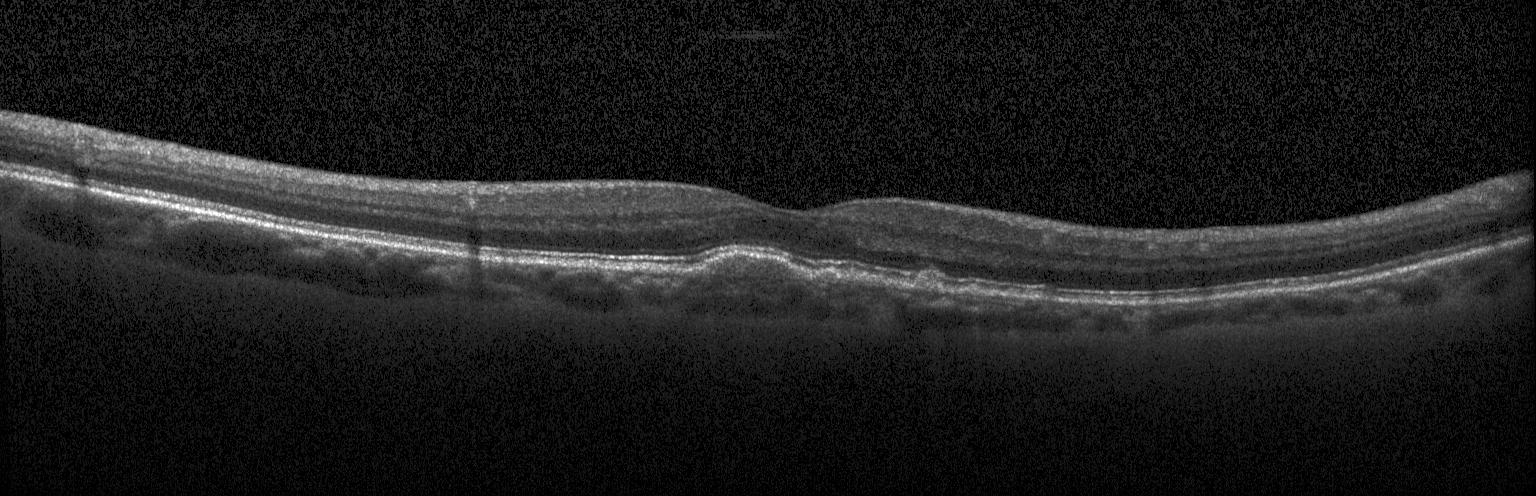 Optical coherence tomography B-scan. Horizontal scan through the fovea. Spectral-domain OCT. Heidelberg Spectralis — Diagnosis: multiple drusen.